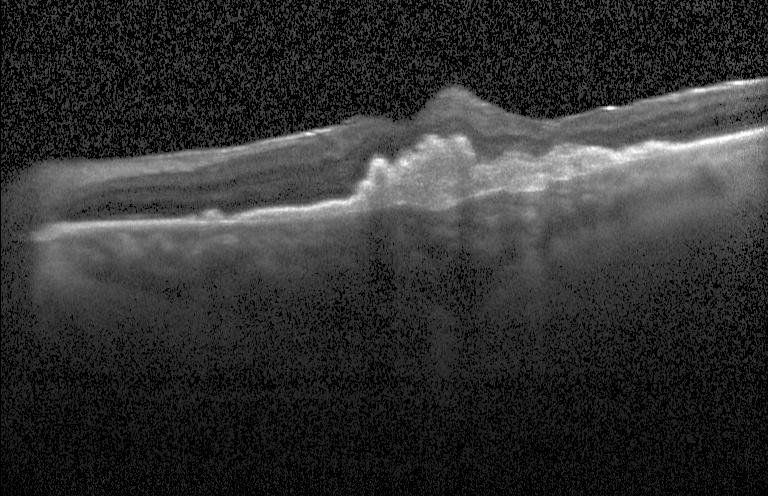
Diagnosis: choroidal neovascularization.